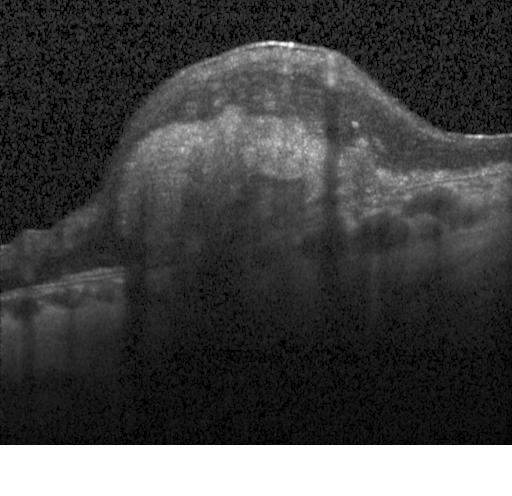
Through the macula; retinal OCT B-scan; acquired on a Heidelberg Spectralis
Diagnosis: choroidal neovascularization.